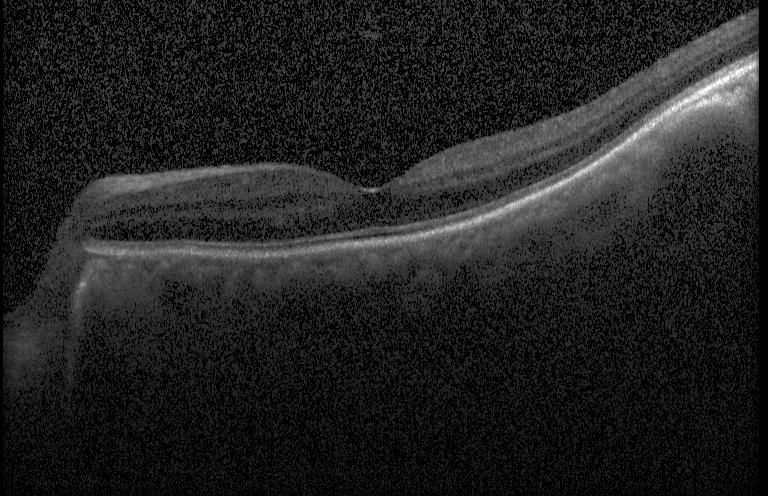

OCT line scan; fovea-centered; instrument: Heidelberg Spectralis — Finding: no CNV, no DME, and no drusen.